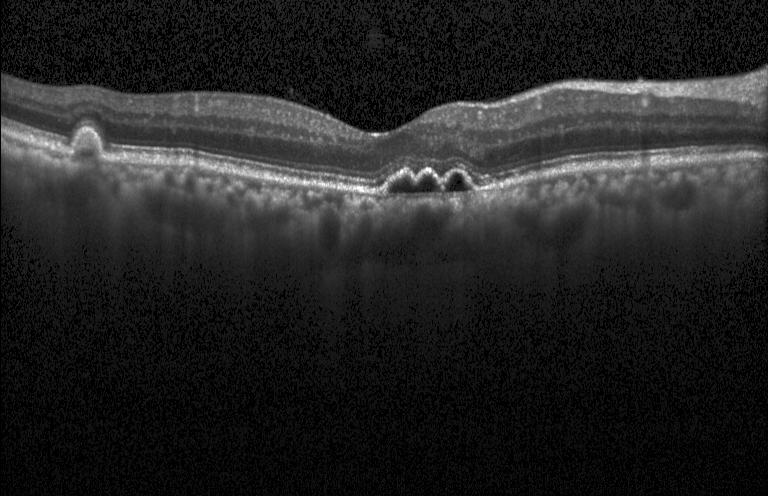 Optical coherence tomography B-scan.
Dx: choroidal neovascularization (CNV).